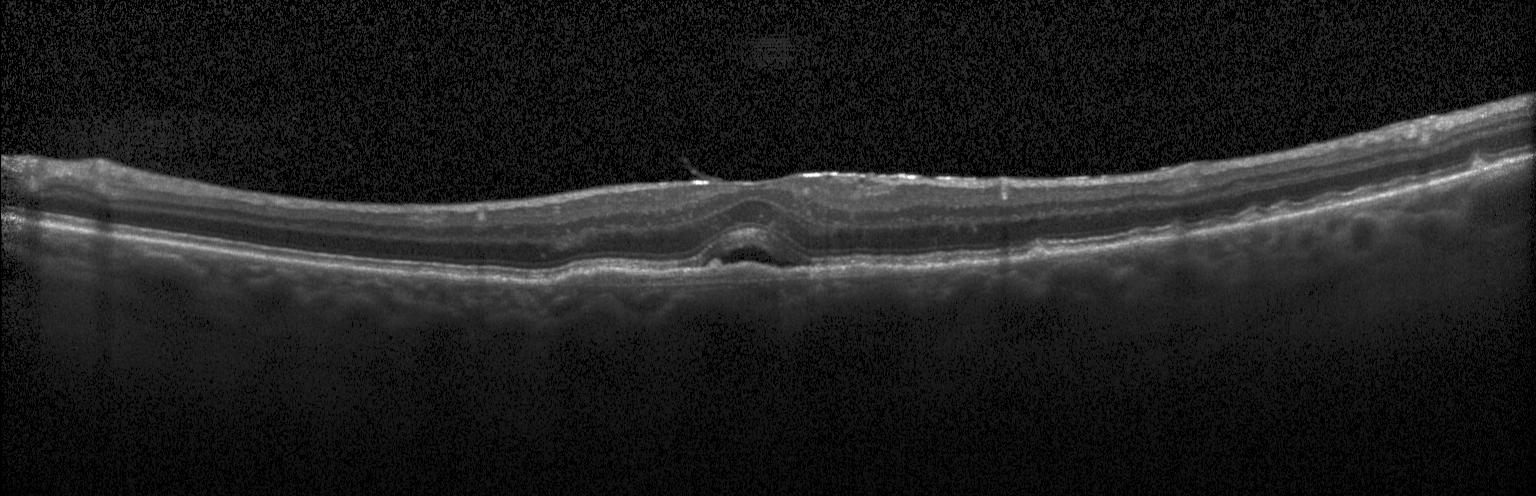 OCT B-scan. Impression: a choroidal neovascular membrane.